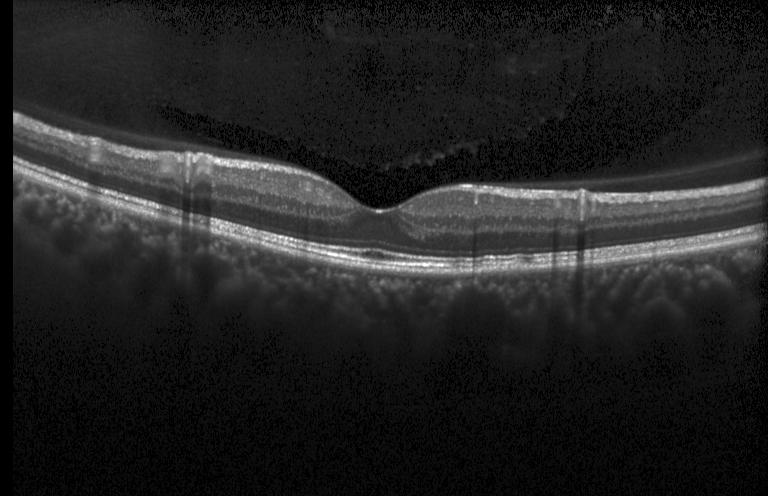 Neither CNV, DME, nor drusen.